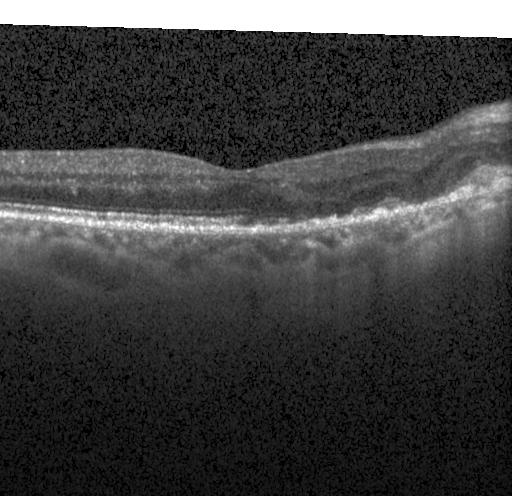
Optical coherence tomography scan.
Macular OCT: choroidal neovascularization.